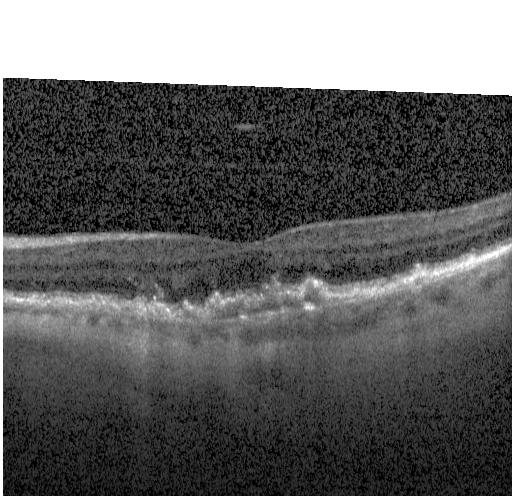

Diagnosis: a choroidal neovascular membrane.